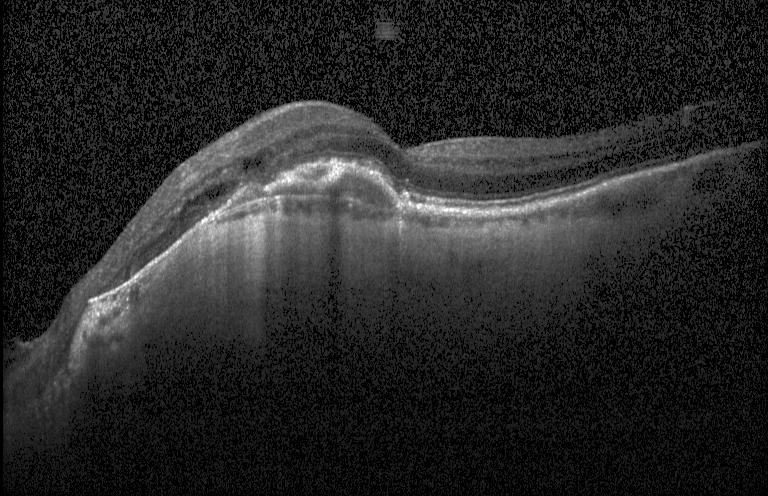
Fovea-centered; optical coherence tomography scan.
Impression: a choroidal neovascular membrane.